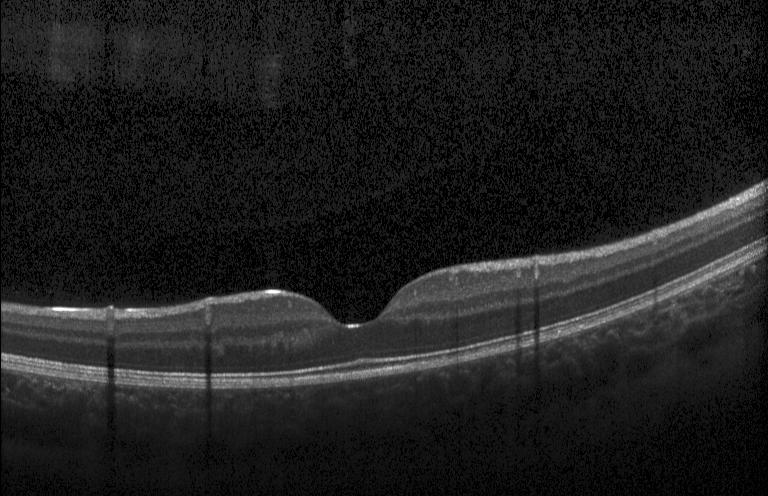 Spectral-domain OCT · OCT B-scan · horizontal scan through the fovea · Heidelberg Spectralis. Assessment: no CNV, DME, or drusen.